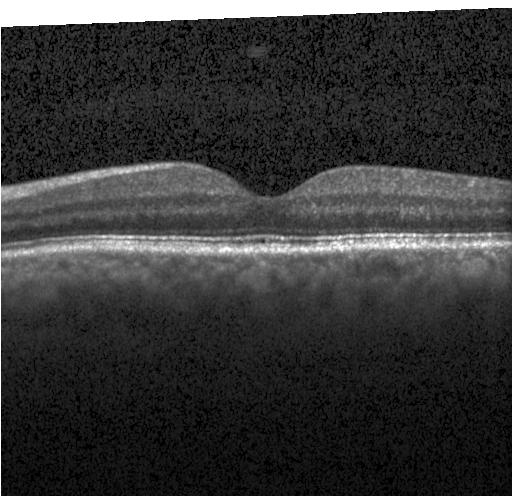 Finding: neither choroidal neovascularization, diabetic macular edema, nor drusen.